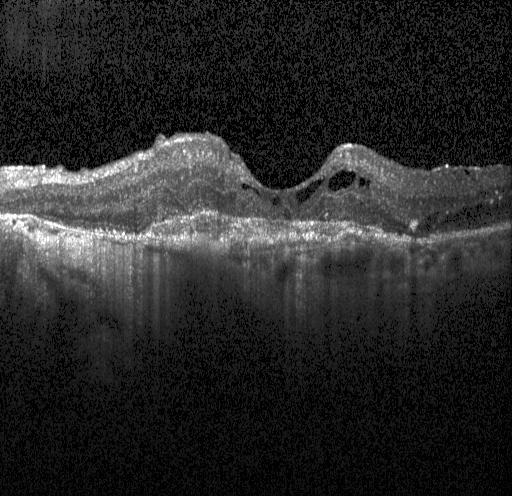
Retinal OCT cross-section.
Assessment: choroidal neovascularization.